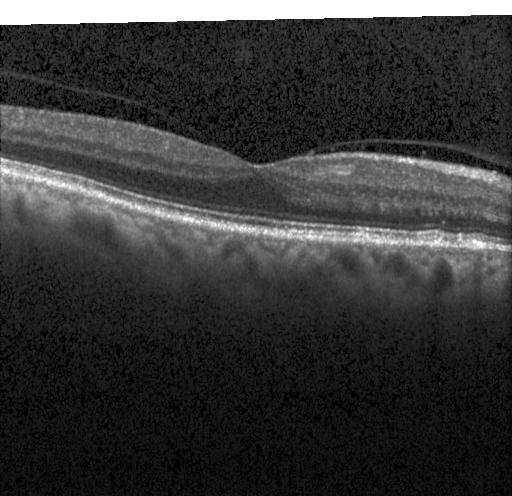 Heidelberg Spectralis OCT system. Spectral-domain optical coherence tomography. OCT B-scan.
Assessment: drusen.